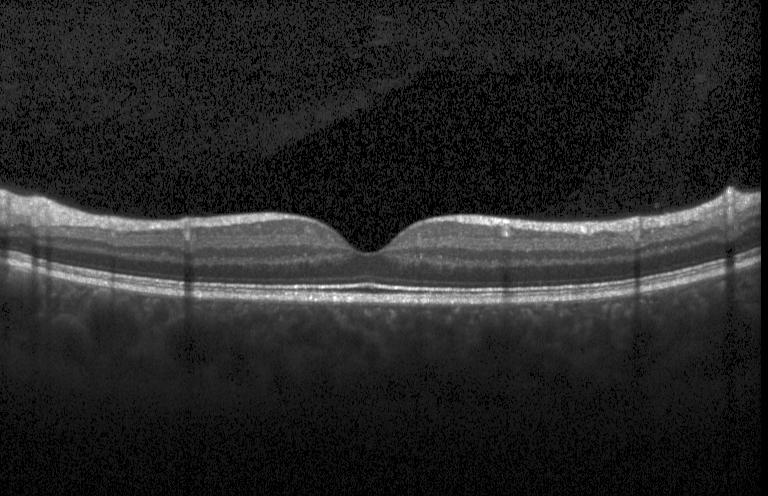

Diagnosis: no choroidal neovascularization, diabetic macular edema, or drusen.